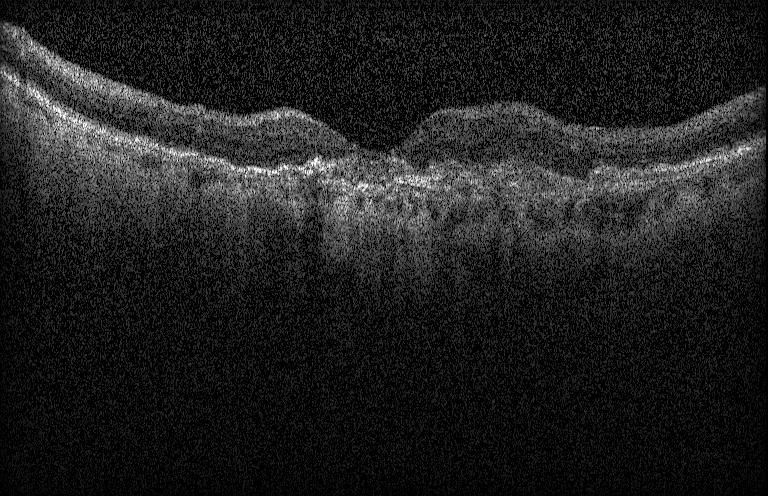

Spectral-domain OCT B-scan: a choroidal neovascular membrane.